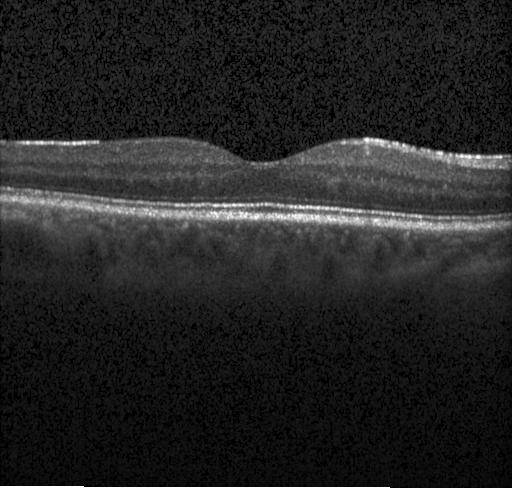 Macular OCT demonstrating neither choroidal neovascularization, diabetic macular edema, nor drusen.